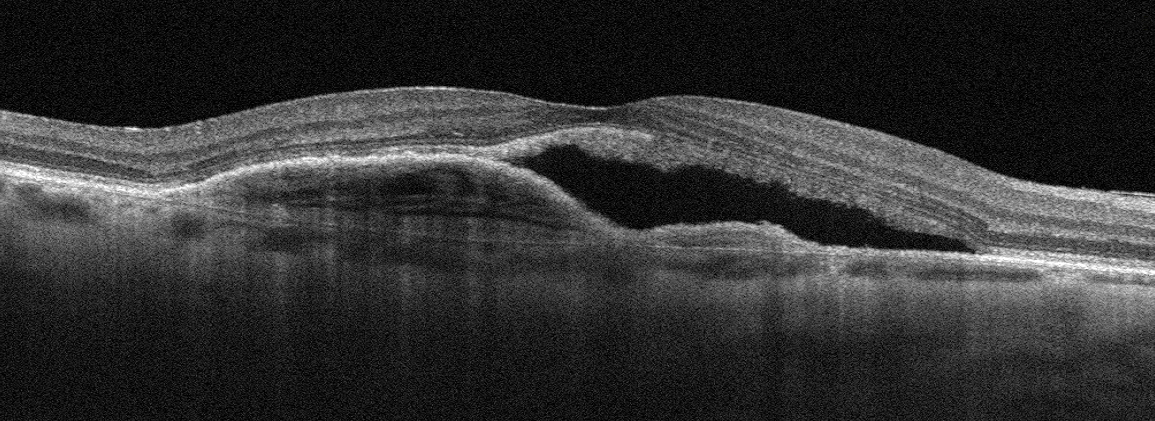 Finding: age-related macular degeneration.